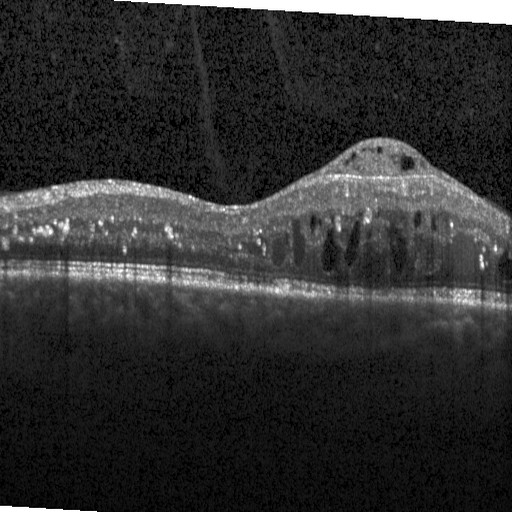 Fovea-centered · SD-OCT · OCT B-scan — Finding: diabetic macular edema.